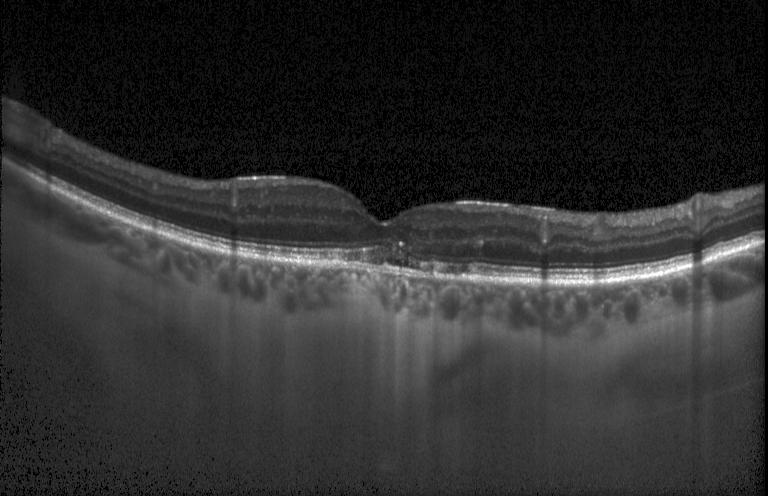
Macular OCT: CNV.